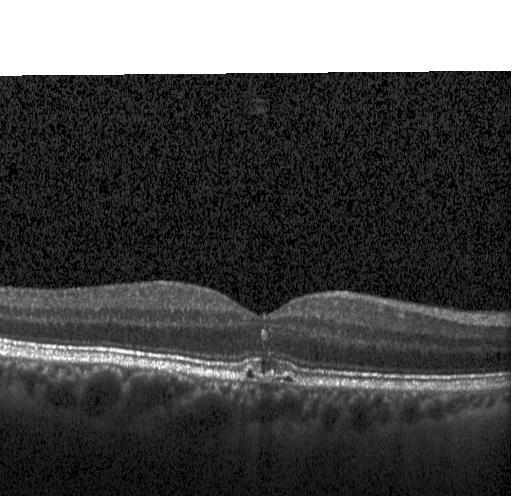 Impression: a choroidal neovascular membrane.